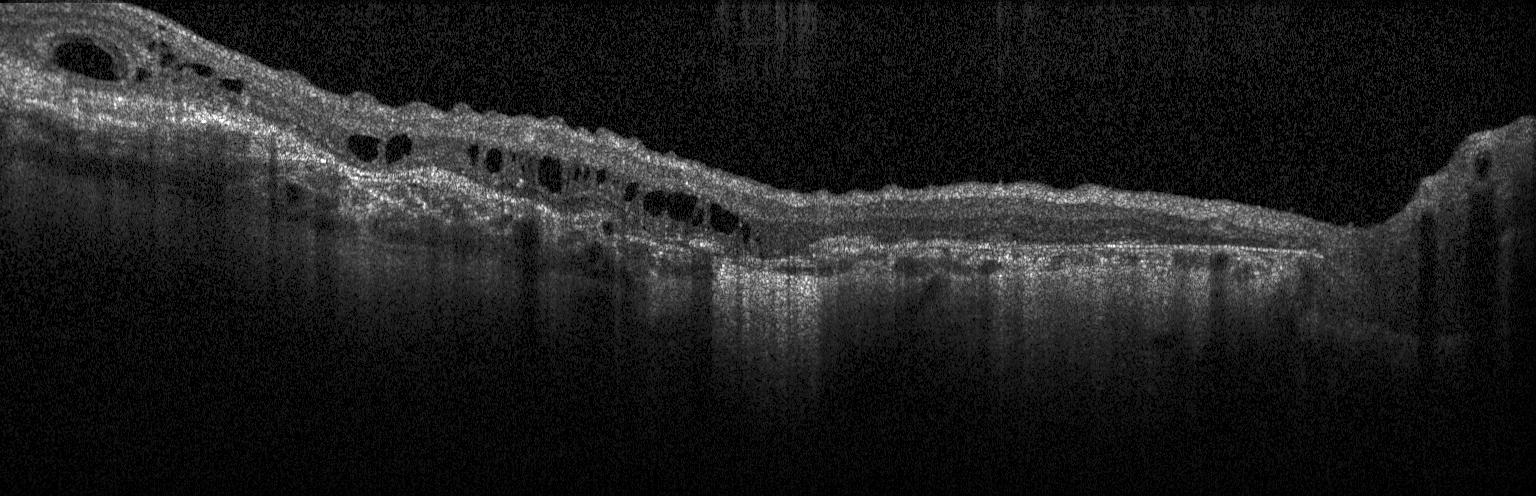 OCT B-scan — Finding: a choroidal neovascular membrane.